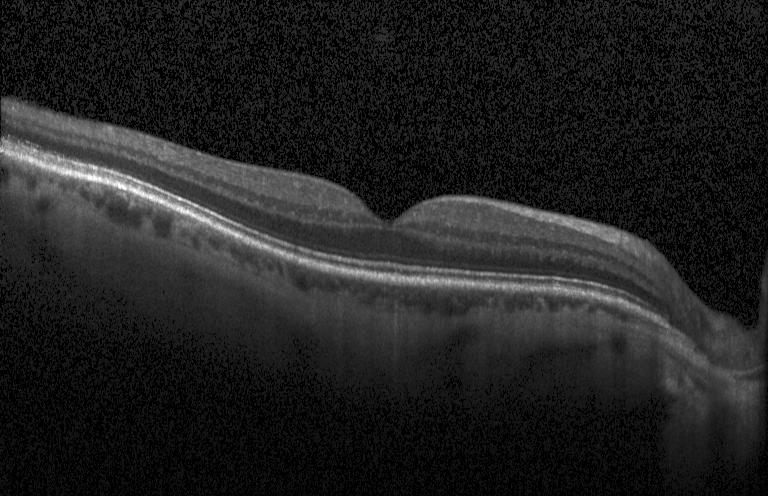 Macular OCT: neither choroidal neovascularization, diabetic macular edema, nor drusen.